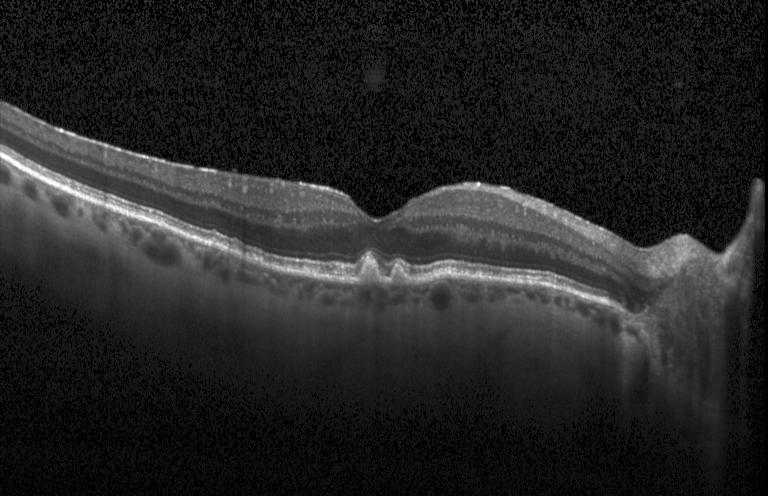 Retinal OCT cross-section showing drusen.